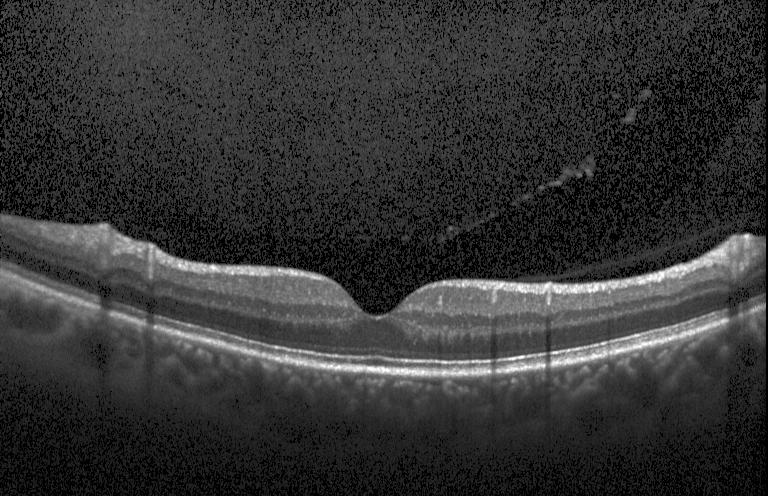
Finding: no choroidal neovascularization, diabetic macular edema, or drusen.